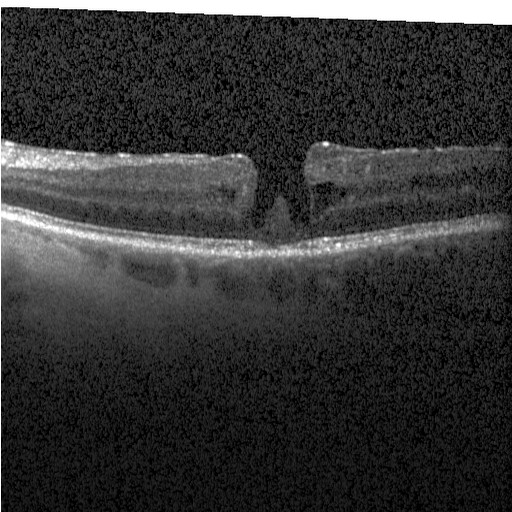 Finding: diabetic macular edema (DME).